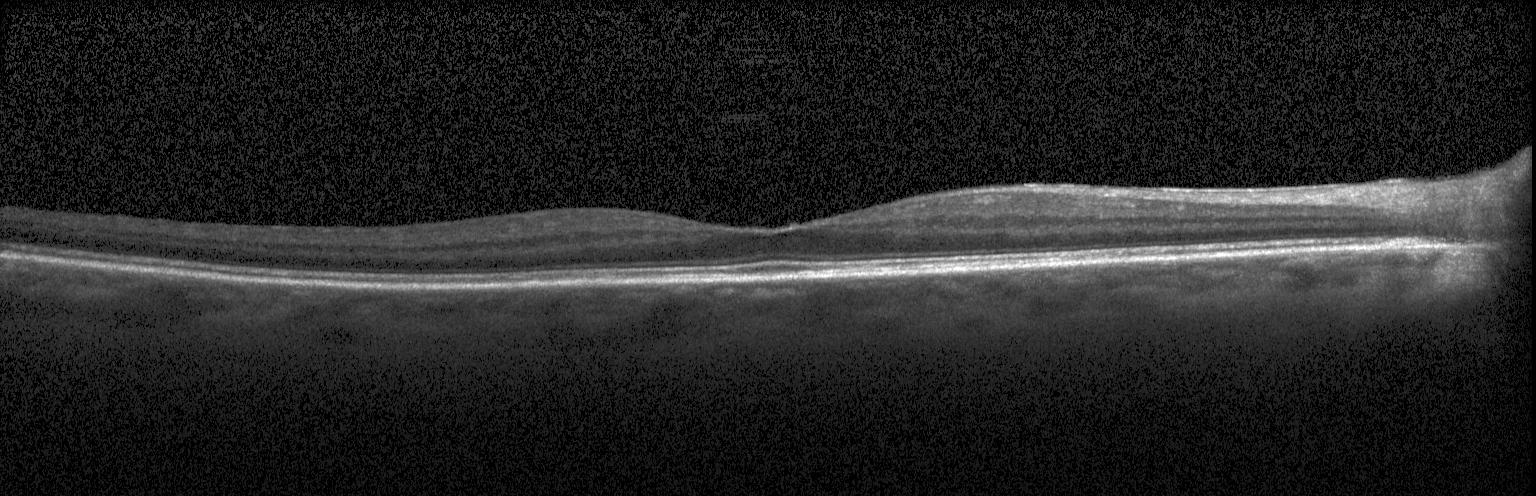
Heidelberg Spectralis OCT system; fovea-centered; spectral-domain optical coherence tomography; retinal OCT B-scan. Finding: neither CNV, DME, nor drusen.